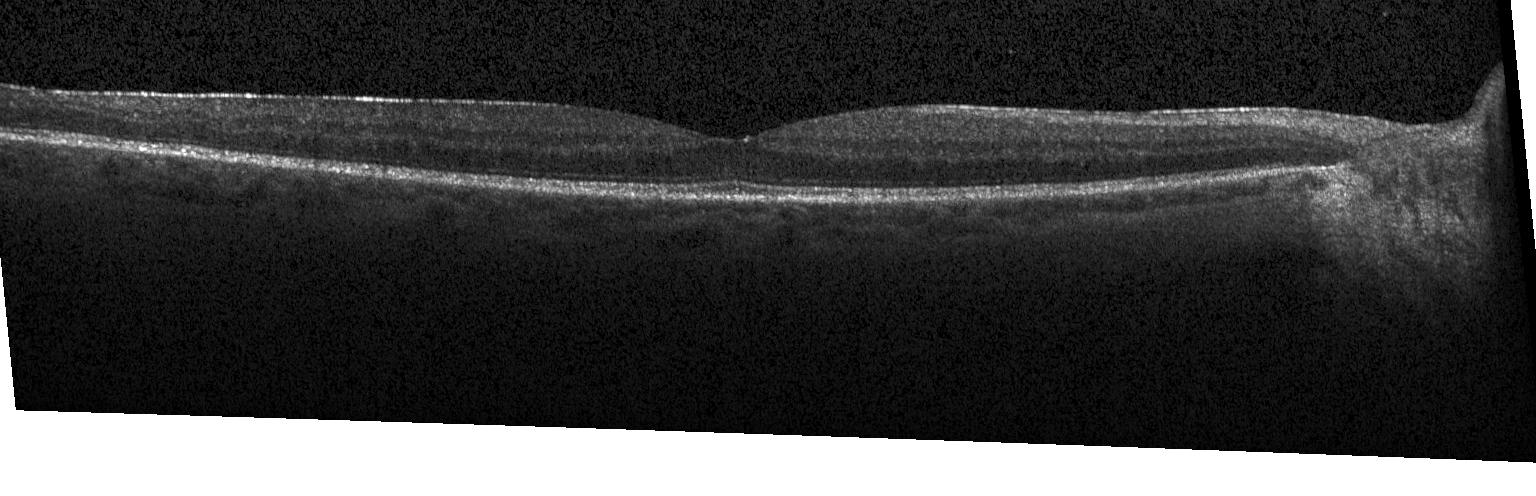 Spectral-domain optical coherence tomography · Heidelberg Spectralis · retinal OCT cross-section. Dx: neither CNV, DME, nor drusen.